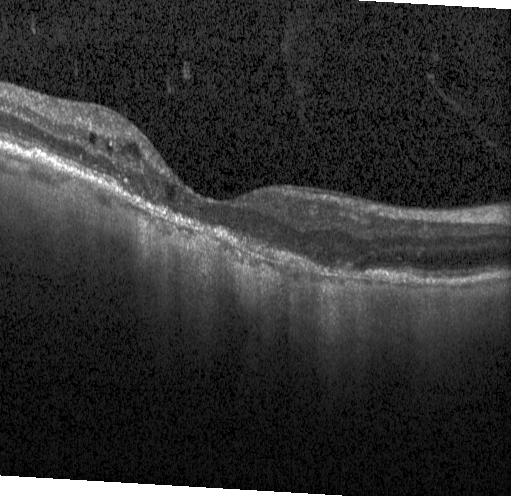

Choroidal neovascularization.